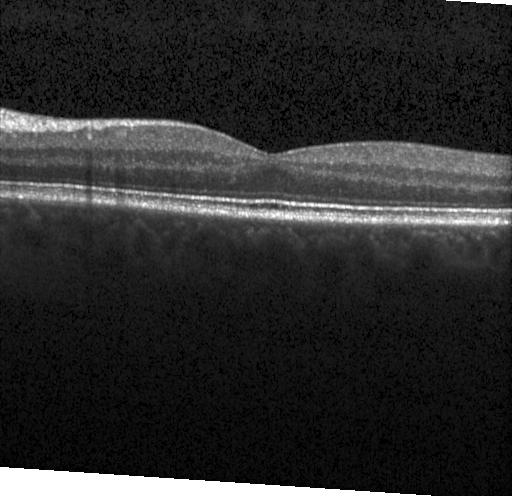

Spectral-domain OCT, OCT B-scan.
Finding: no choroidal neovascularization, no diabetic macular edema, and no drusen.